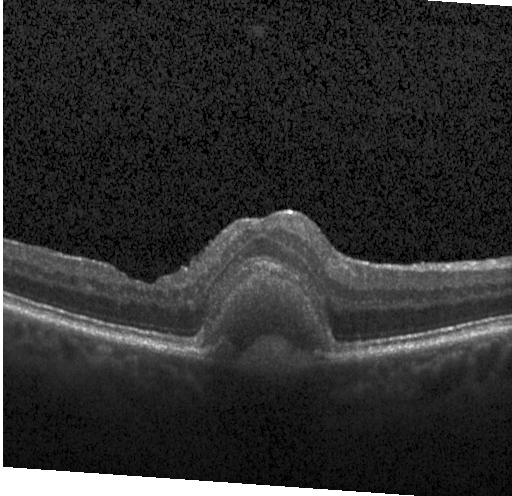 Centered on the fovea; OCT line scan.
Diagnosis: choroidal neovascularization.